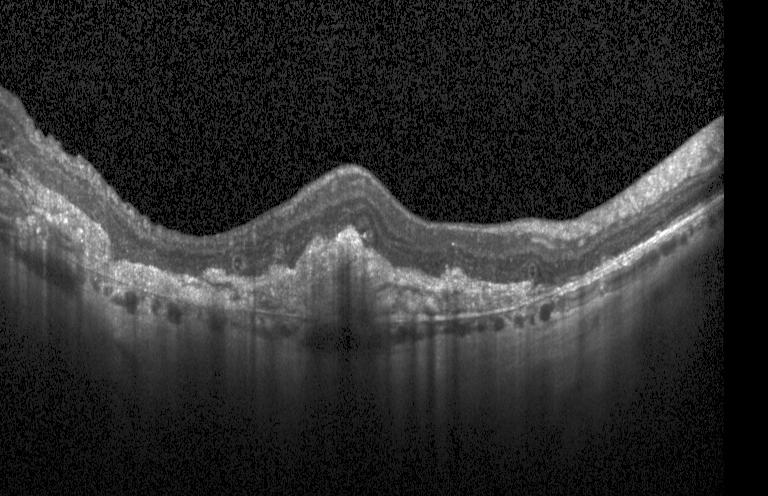 Dx: a choroidal neovascular membrane.